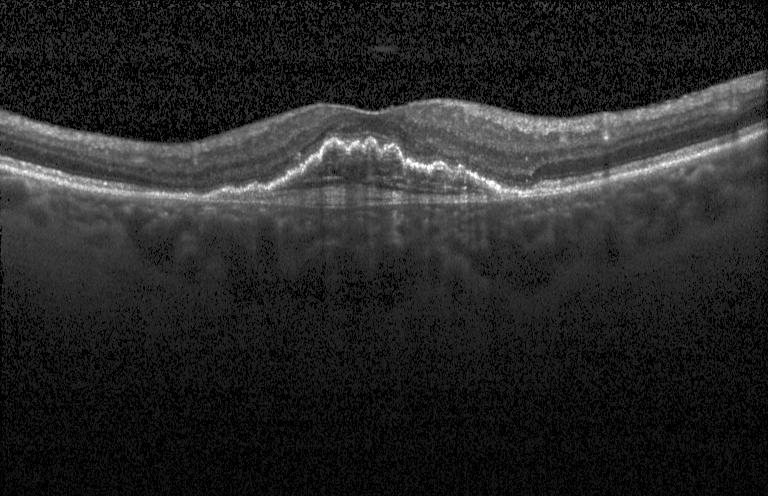 Diagnosis: a choroidal neovascular membrane.